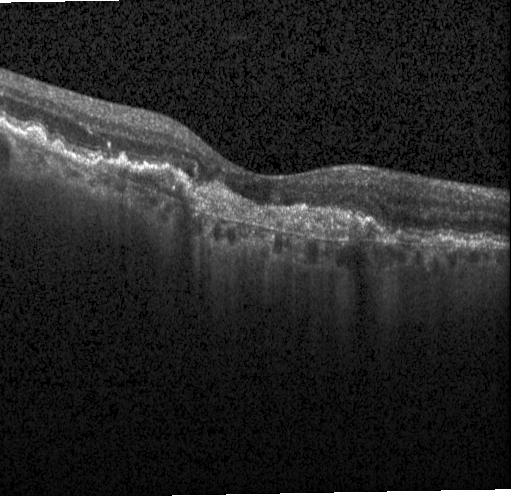
Diagnosis: choroidal neovascularization.